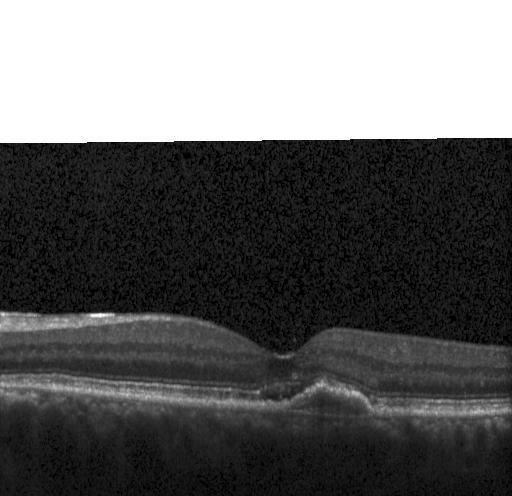

OCT B-scan showing choroidal neovascularization (CNV).